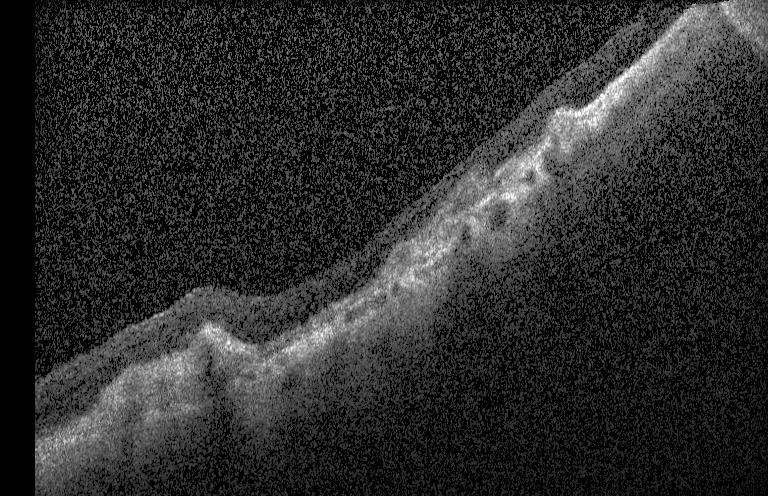

Through the macula; spectral-domain OCT; Heidelberg Spectralis OCT system; OCT line scan. Finding: a choroidal neovascular membrane.